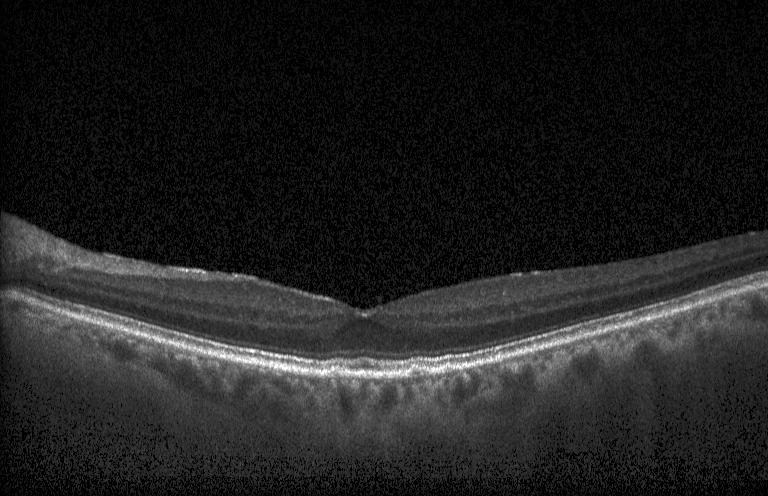
Macular OCT demonstrating drusen.